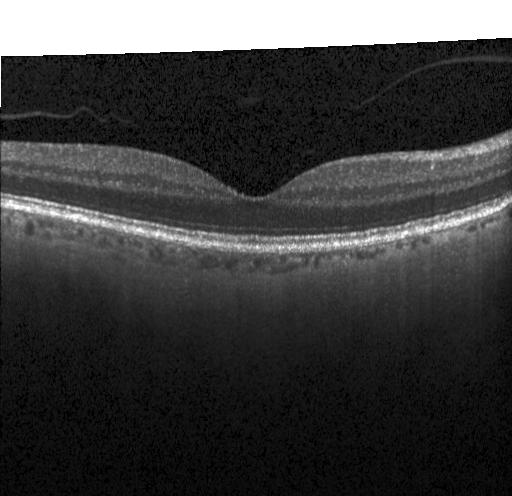
Through the macula · spectral-domain optical coherence tomography · OCT B-scan.
Impression: no evidence of choroidal neovascularization, diabetic macular edema, or drusen.